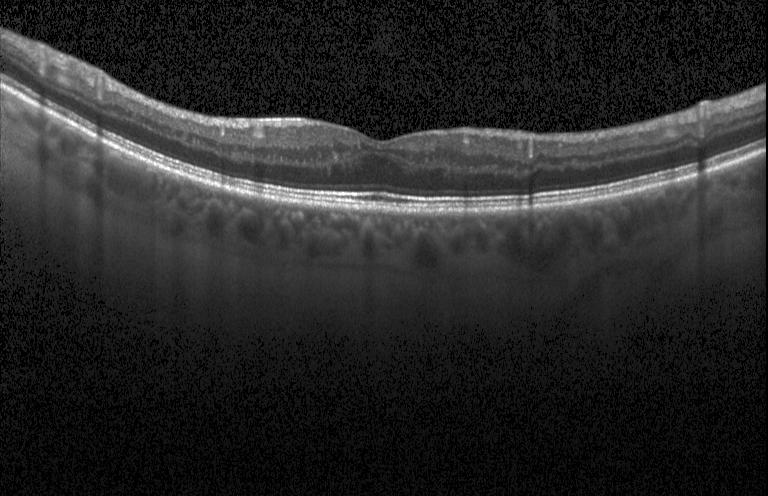
SD-OCT, macular scan, retinal OCT cross-section — Diagnosis: neither choroidal neovascularization, diabetic macular edema, nor drusen.